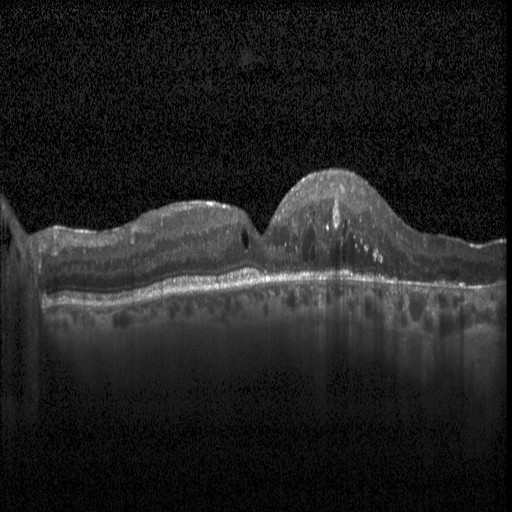
Optical coherence tomography B-scan.
Diagnosis: diabetic macular edema.